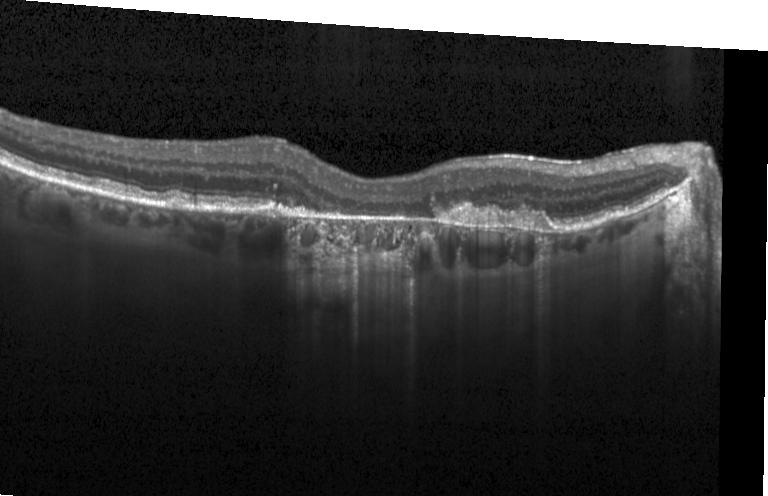 Impression: choroidal neovascularization.